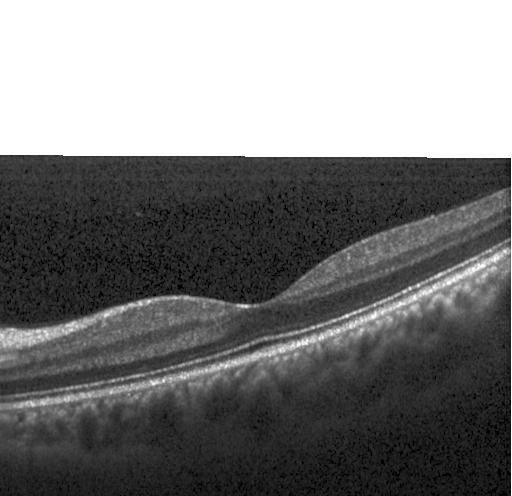
Spectral-domain OCT · optical coherence tomography B-scan. OCT finding: no choroidal neovascularization, no diabetic macular edema, and no drusen.